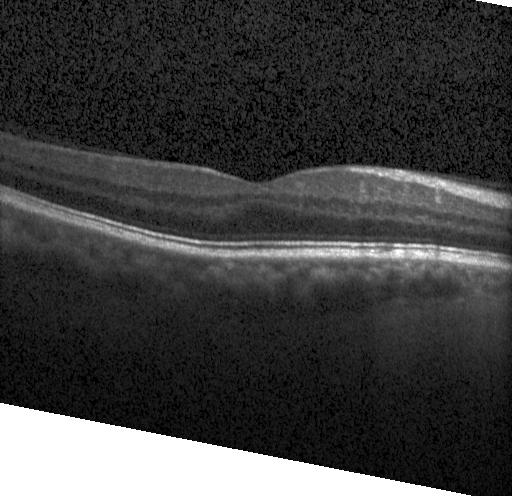 Through the macula, optical coherence tomography scan, spectral-domain OCT, acquired on a Heidelberg Spectralis
Impression: neither CNV, DME, nor drusen.